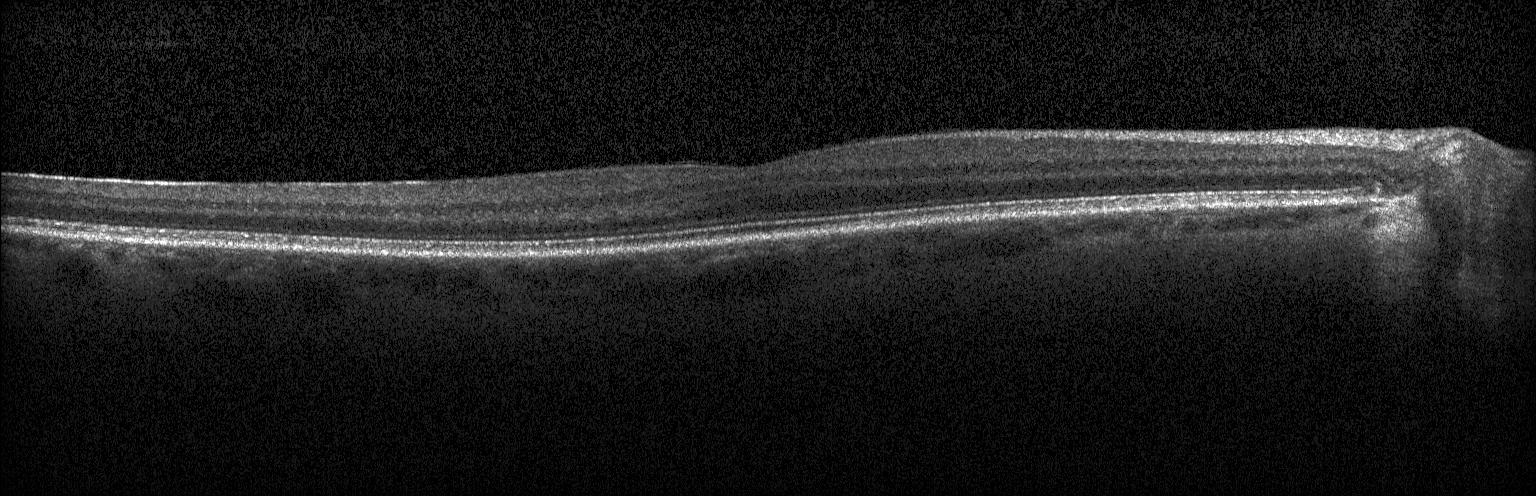
Finding: no CNV, no DME, and no drusen.